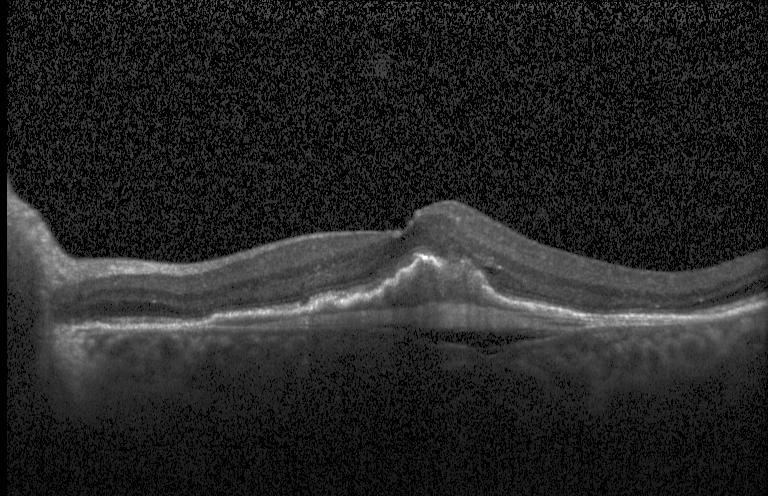
Dx: CNV.